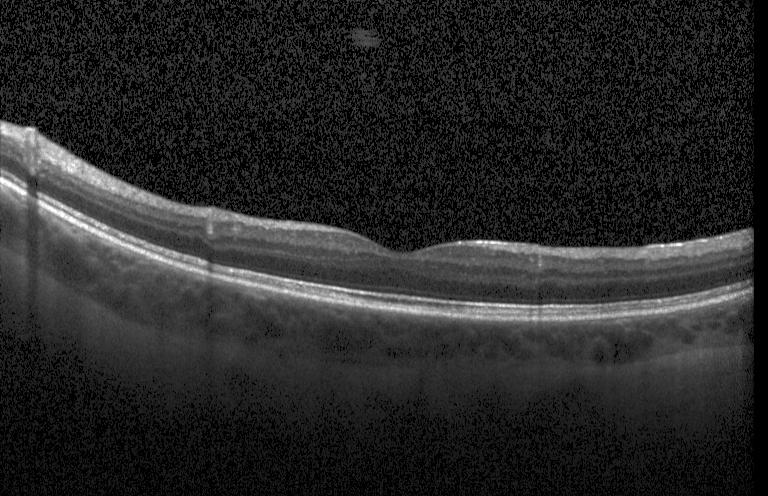 Spectral-domain optical coherence tomography · acquired on a Heidelberg Spectralis · fovea-centered · retinal OCT cross-section
Impression: no evidence of choroidal neovascularization, diabetic macular edema, or drusen.